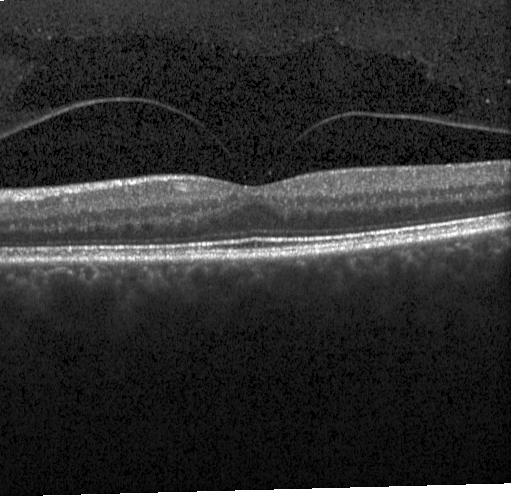
OCT finding: no evidence of CNV, DME, or drusen.